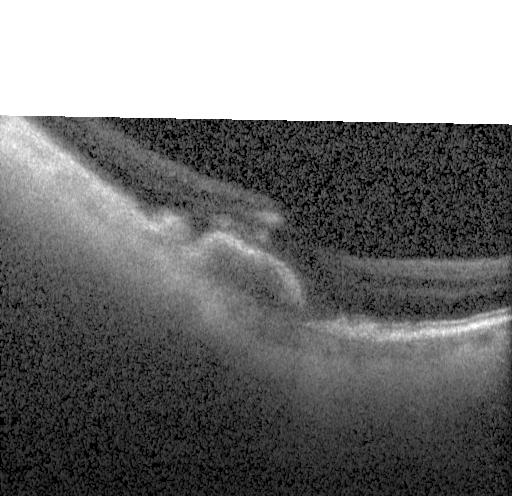
Impression: a choroidal neovascular membrane.